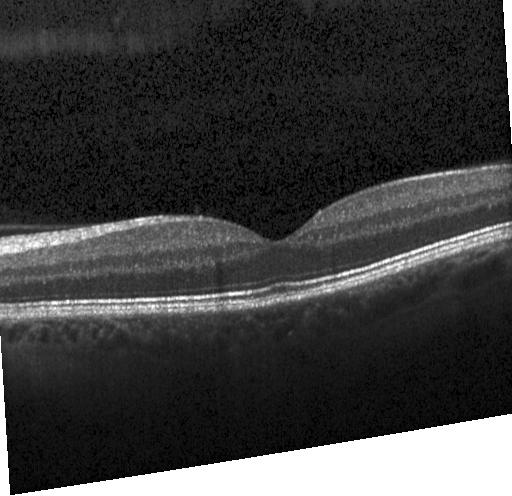

OCT B-scan; Heidelberg Spectralis.
OCT finding: no evidence of choroidal neovascularization, diabetic macular edema, or drusen.